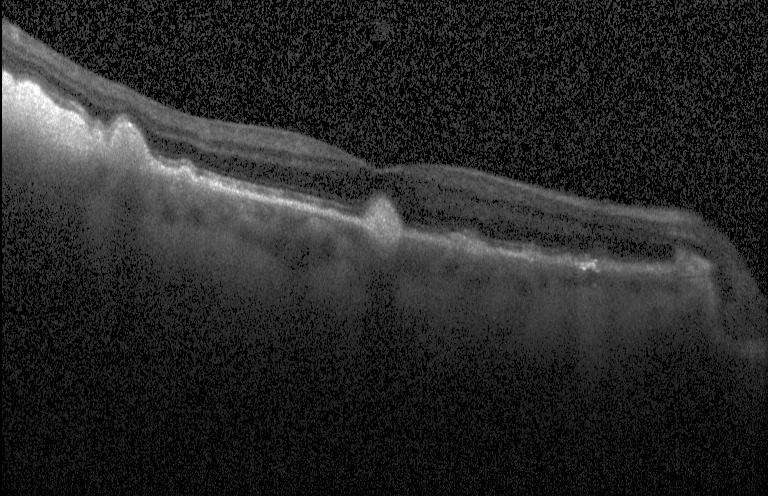
OCT B-scan.
Finding: multiple drusen.